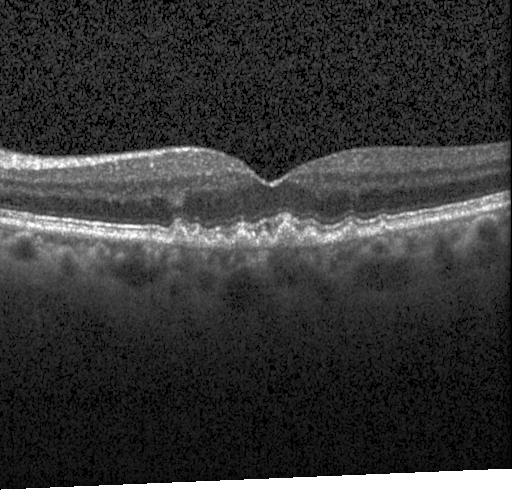 SD-OCT, centered on the fovea, retinal OCT cross-section
Assessment: multiple drusen.